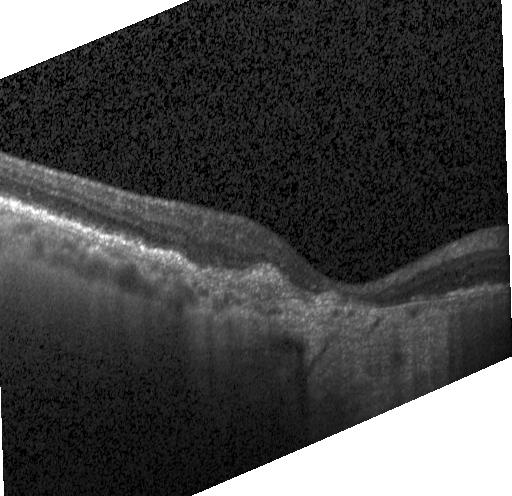
OCT scan showing a choroidal neovascular membrane.